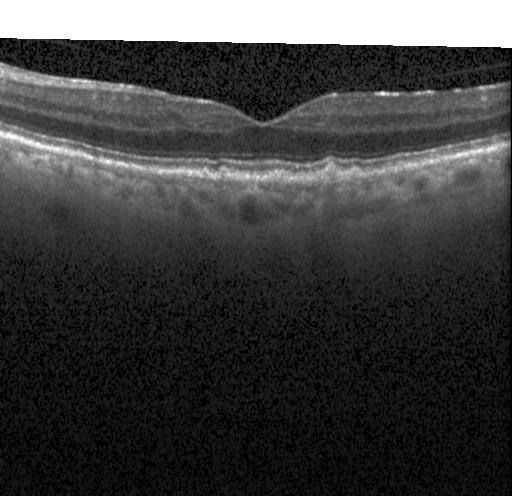

Macular scan, optical coherence tomography B-scan, spectral-domain optical coherence tomography, Heidelberg Spectralis — Assessment: sub-RPE drusenoid deposits.